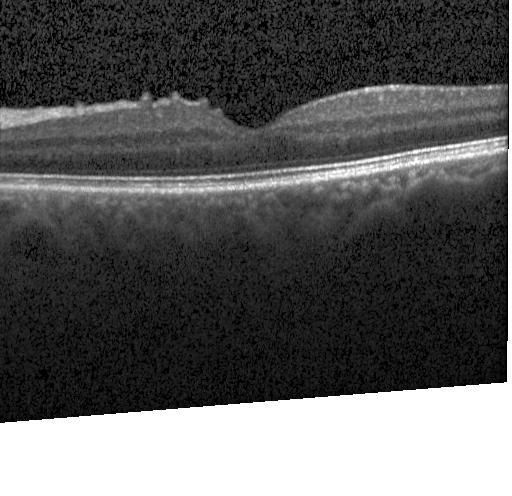 OCT line scan, SD-OCT, fovea-centered. The scan shows neither choroidal neovascularization, diabetic macular edema, nor drusen.